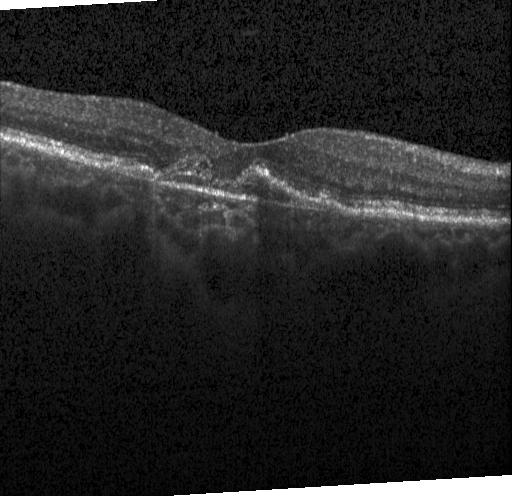 Heidelberg Spectralis, fovea-centered, SD-OCT, optical coherence tomography scan.
Diagnosis: CNV.